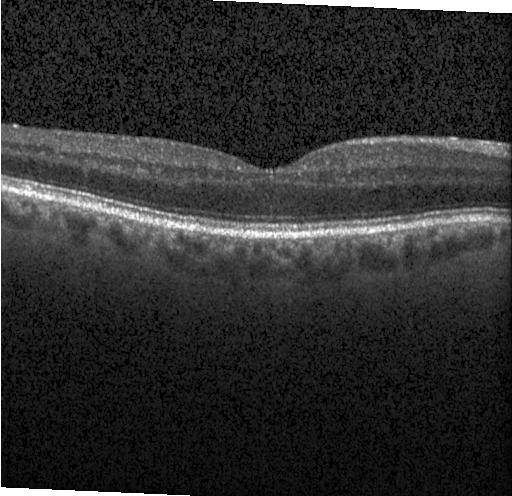
Retinal OCT B-scan
Impression: no choroidal neovascularization, no diabetic macular edema, and no drusen.